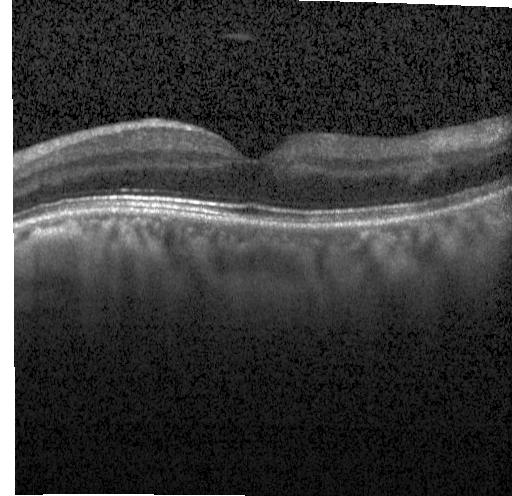 Dx: no choroidal neovascularization, diabetic macular edema, or drusen.